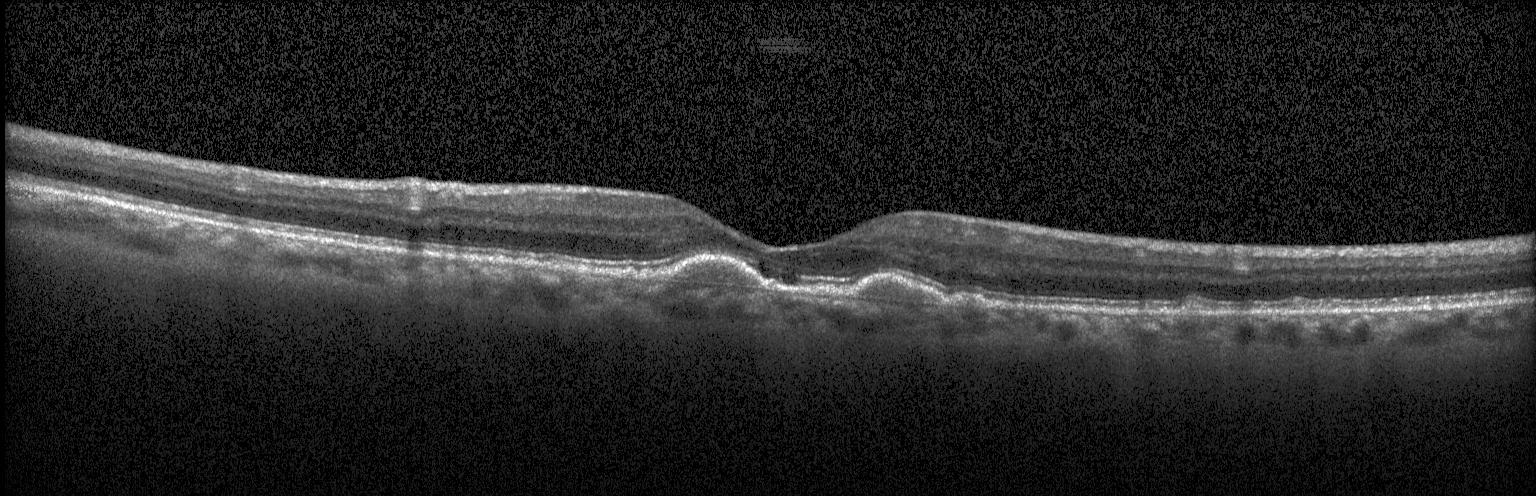 Instrument: Heidelberg Spectralis; optical coherence tomography B-scan. Dx: drusen.